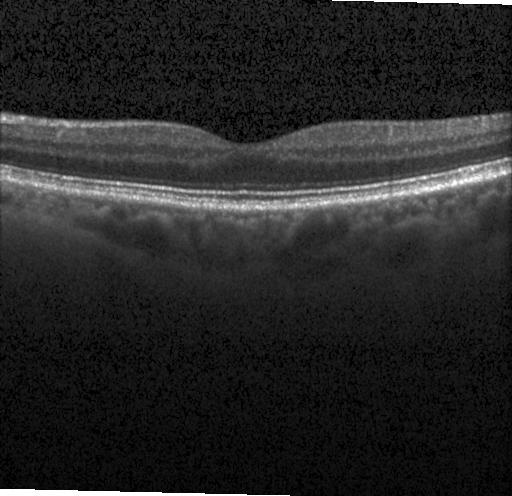 The scan shows no choroidal neovascularization, no diabetic macular edema, and no drusen.